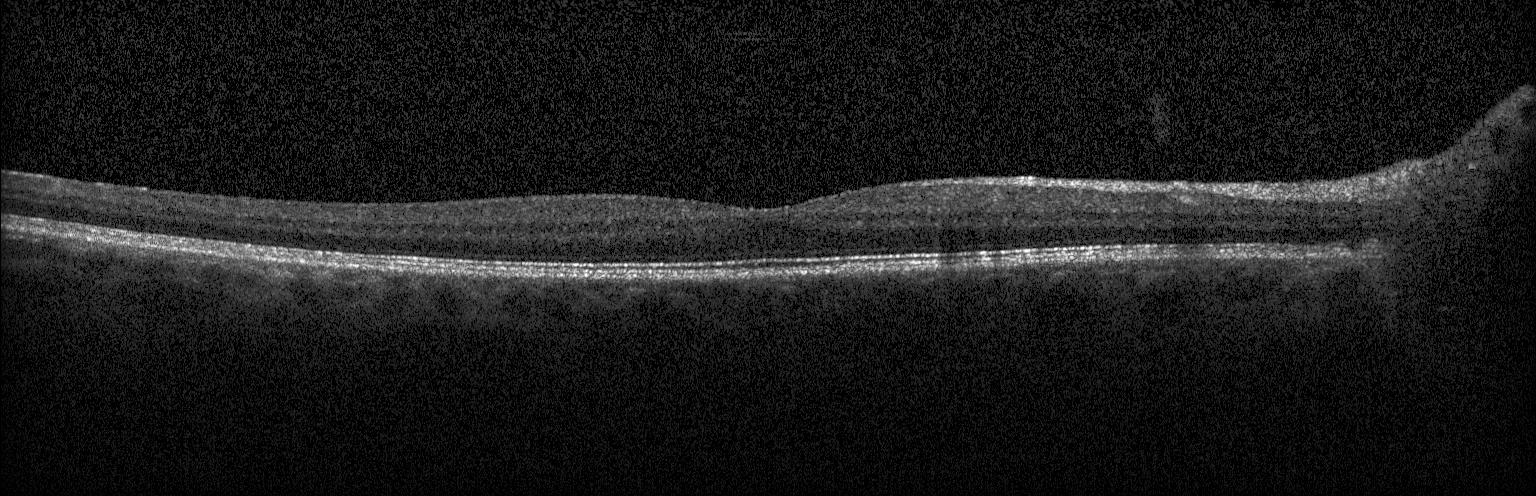

This B-scan demonstrates no evidence of CNV, DME, or drusen.